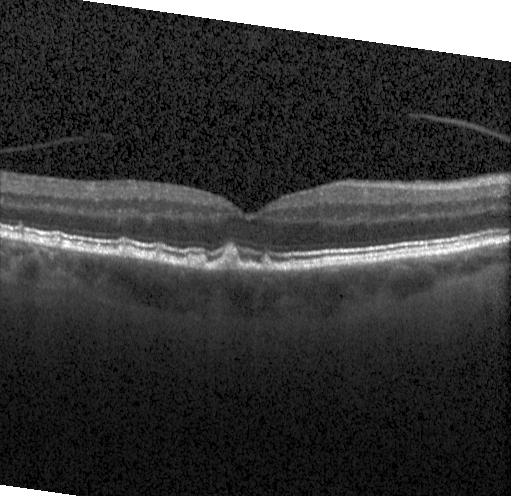

OCT scan showing drusen.